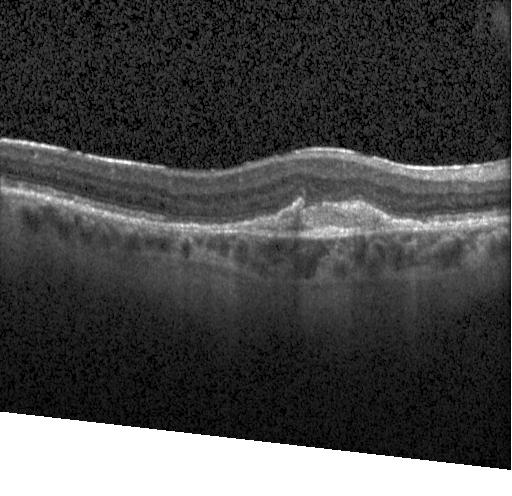

Spectral-domain OCT · OCT B-scan
This B-scan demonstrates choroidal neovascularization.